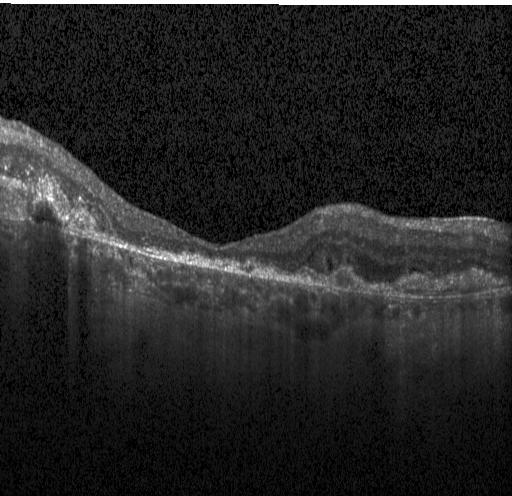
Optical coherence tomography scan — A choroidal neovascular membrane.